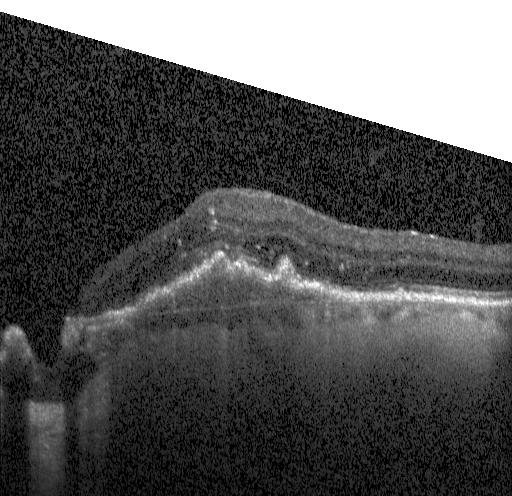 Acquired on a Heidelberg Spectralis, retinal OCT cross-section — This B-scan demonstrates CNV.